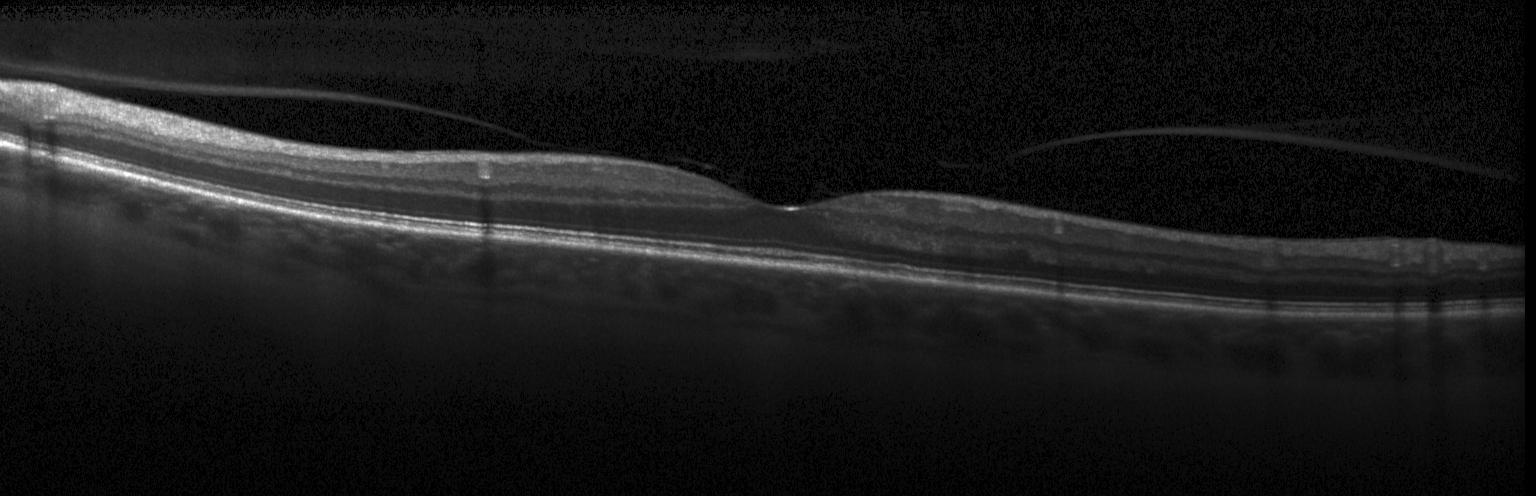

OCT B-scan · instrument: Heidelberg Spectralis · SD-OCT · horizontal scan through the fovea.
Diagnosis: neither CNV, DME, nor drusen.